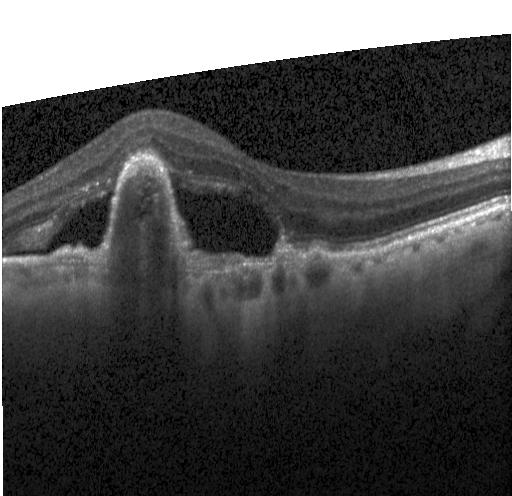

Macular scan. OCT line scan — This B-scan demonstrates CNV.